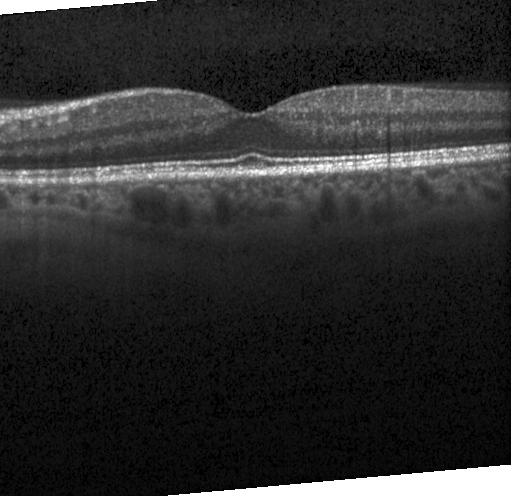 OCT B-scan · centered on the fovea. Dx: no evidence of choroidal neovascularization, diabetic macular edema, or drusen.